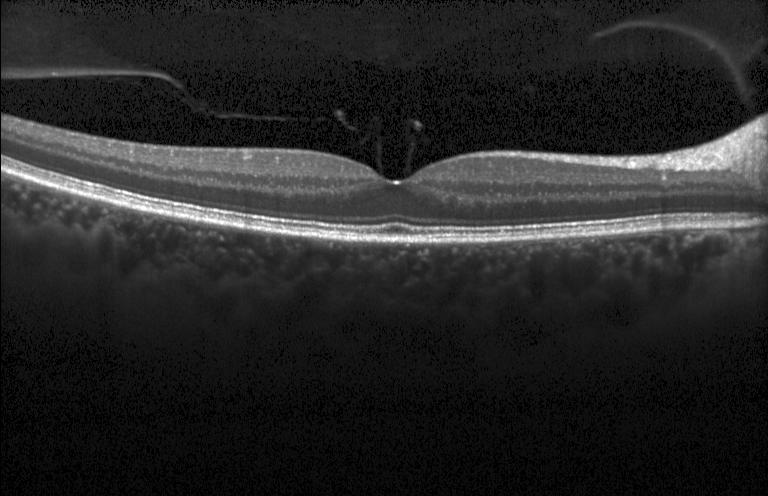 Acquired on a Heidelberg Spectralis, spectral-domain optical coherence tomography, optical coherence tomography scan, centered on the fovea
Diagnosis: neither choroidal neovascularization, diabetic macular edema, nor drusen.